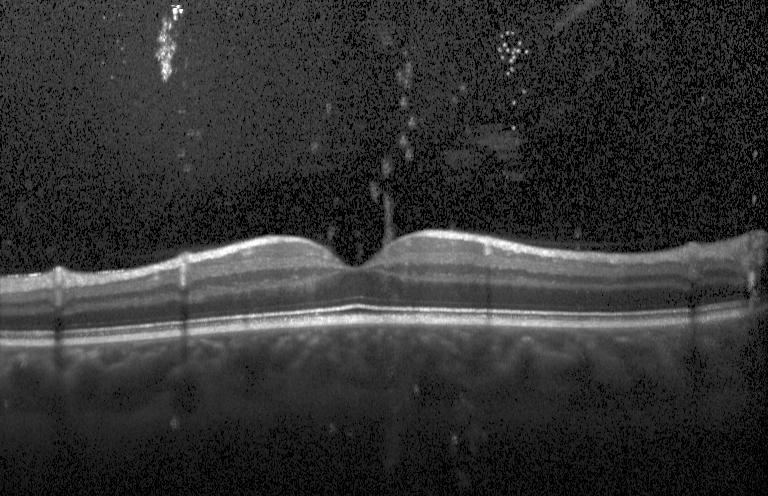
Impression: neither CNV, DME, nor drusen.